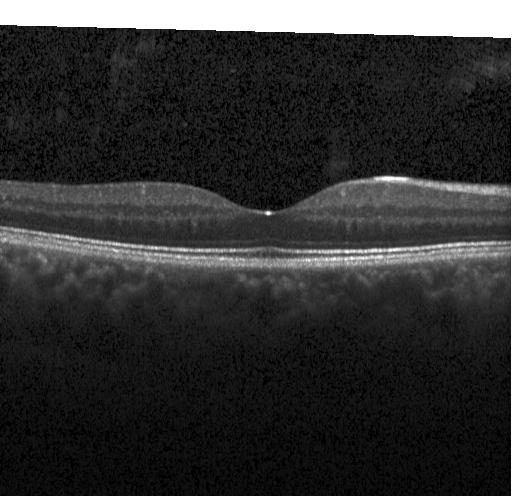 Retinal OCT cross-section.
Diagnosis: no CNV, no DME, and no drusen.